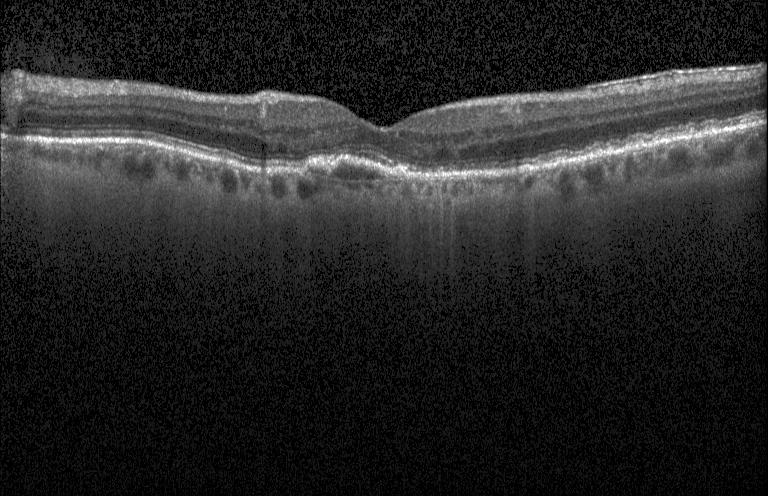

Impression: a choroidal neovascular membrane.